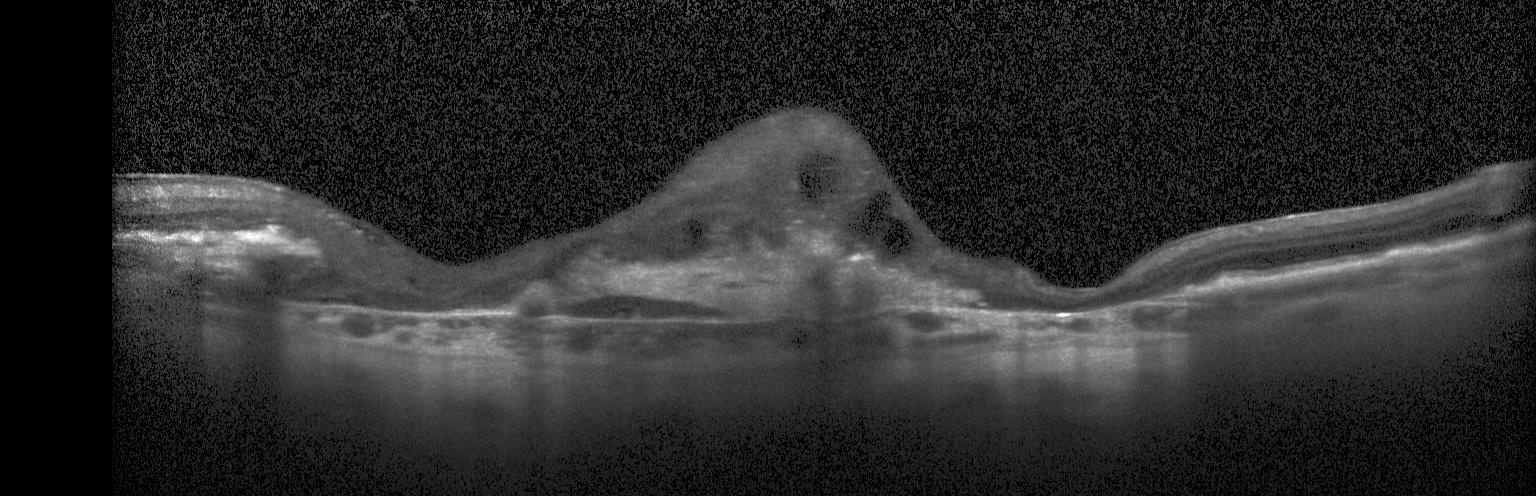
Acquired on a Heidelberg Spectralis; OCT B-scan.
Finding: a choroidal neovascular membrane.